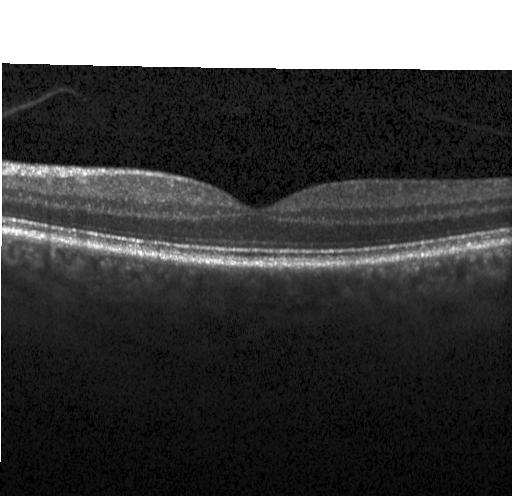 OCT scan showing neither choroidal neovascularization, diabetic macular edema, nor drusen.